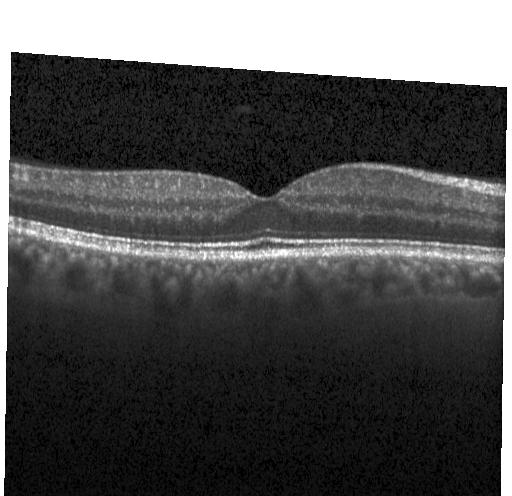
OCT line scan — Finding: no choroidal neovascularization, no diabetic macular edema, and no drusen.